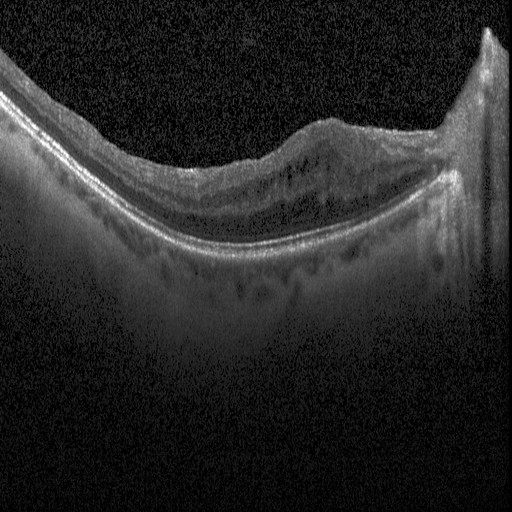

Impression: diabetic macular edema (DME).